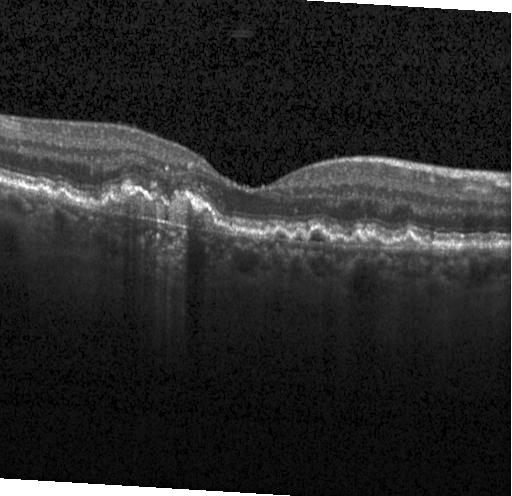 Impression: choroidal neovascularization.